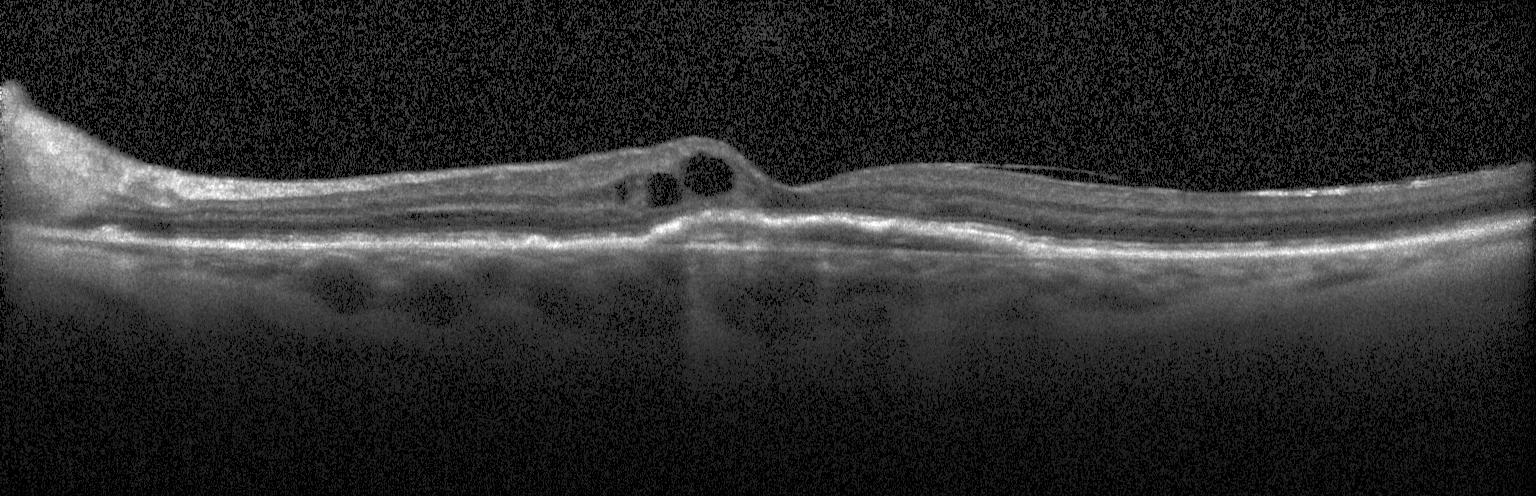 Retinal OCT B-scan; spectral-domain OCT; macular scan — This B-scan demonstrates CNV.